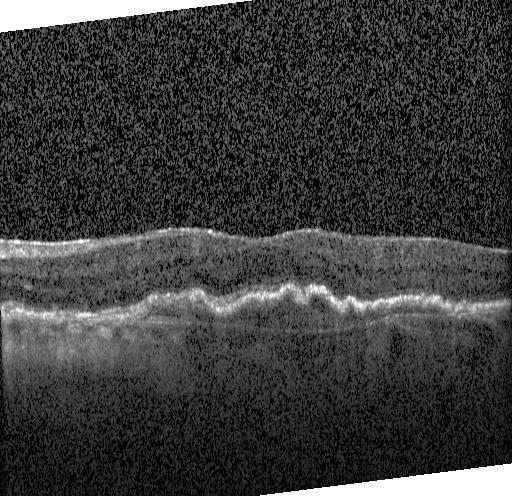 Acquired on a Heidelberg Spectralis. OCT line scan. Fovea-centered. Spectral-domain optical coherence tomography — Choroidal neovascularization.